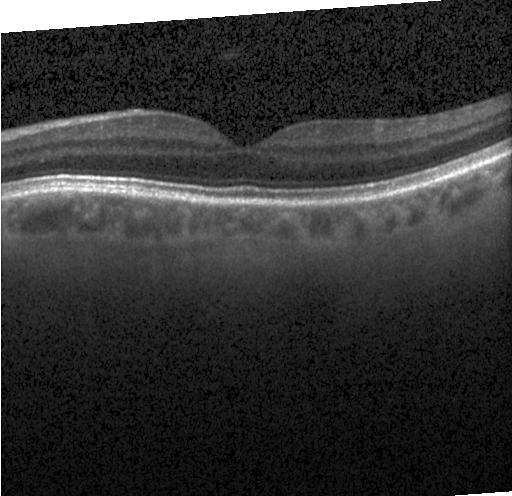
Retinal OCT B-scan — Finding: no choroidal neovascularization, no diabetic macular edema, and no drusen.